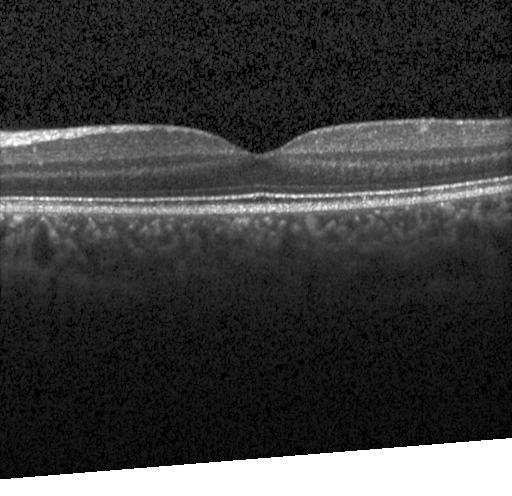
Optical coherence tomography scan; acquired on a Heidelberg Spectralis; horizontal scan through the fovea.
Diagnosis: neither choroidal neovascularization, diabetic macular edema, nor drusen.